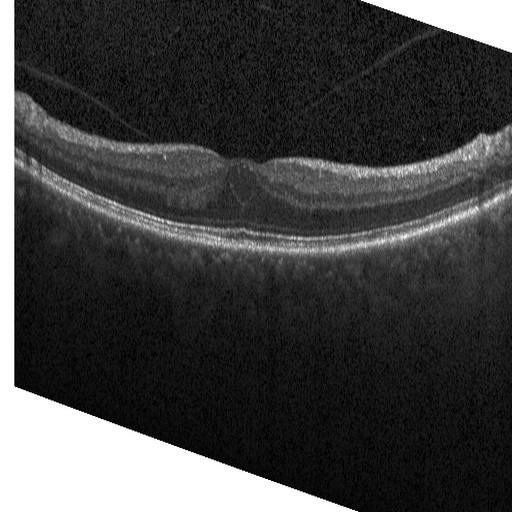 Fovea-centered · optical coherence tomography B-scan.
Diagnosis: diabetic macular edema.